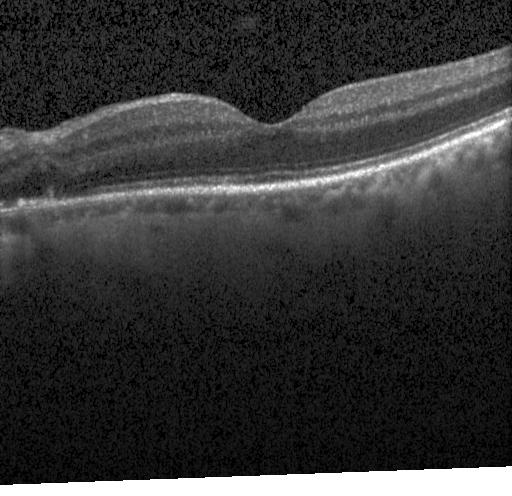
Retinal OCT B-scan · Heidelberg Spectralis OCT system
Diagnosis: no choroidal neovascularization, diabetic macular edema, or drusen.